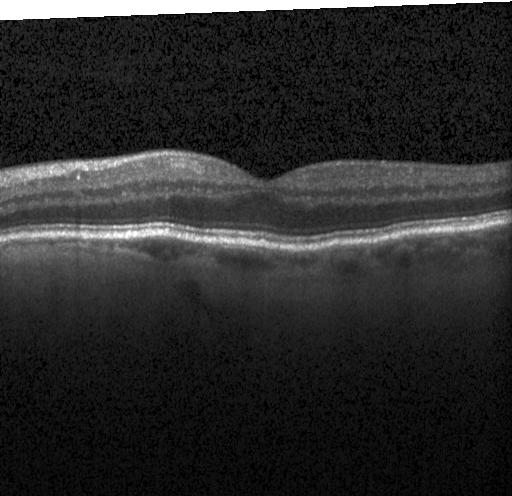 Retinal OCT cross-section.
Macular OCT: no choroidal neovascularization, diabetic macular edema, or drusen.